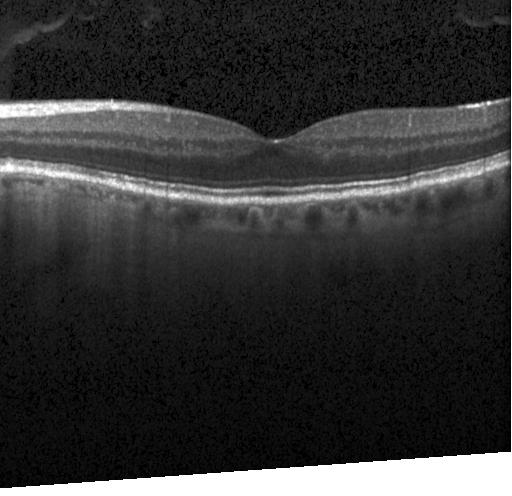

Retinal OCT cross-section showing no CNV, no DME, and no drusen.